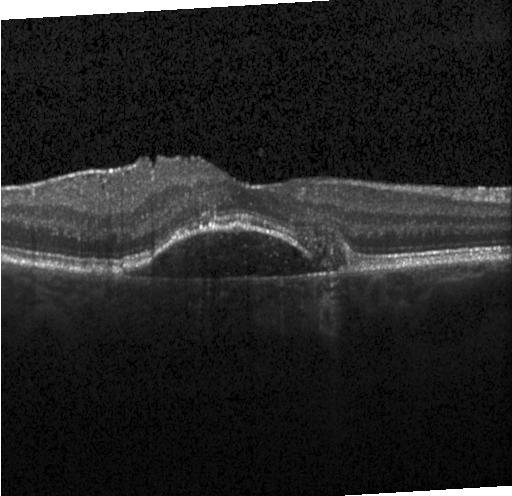

Retinal OCT cross-section. This B-scan demonstrates CNV.